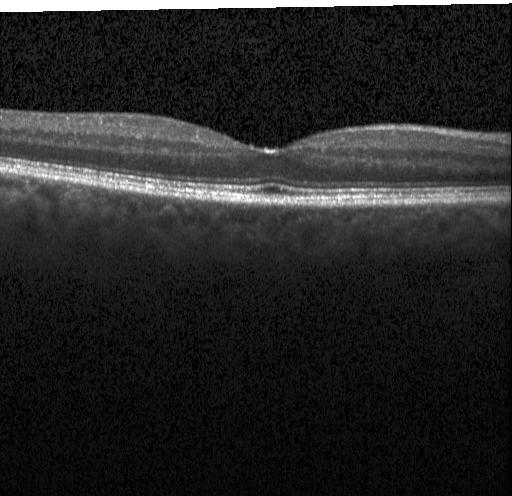

Finding: no evidence of choroidal neovascularization, diabetic macular edema, or drusen.